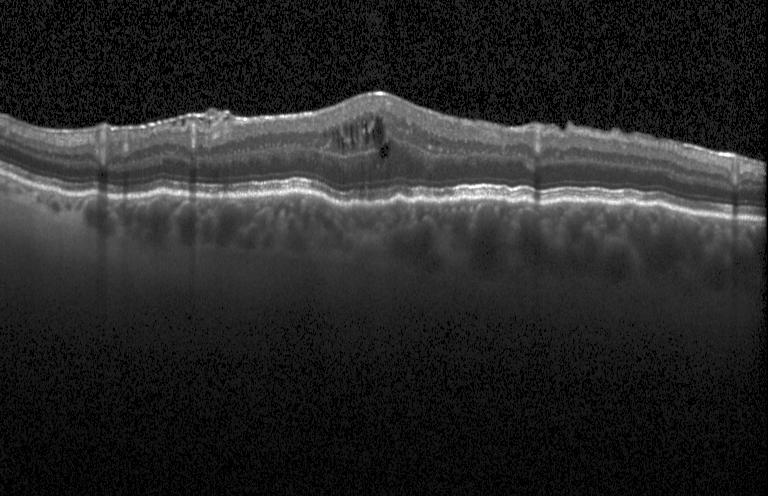
Spectral-domain optical coherence tomography, Heidelberg Spectralis OCT system, horizontal scan through the fovea, retinal OCT cross-section. OCT finding: diabetic macular edema (DME).